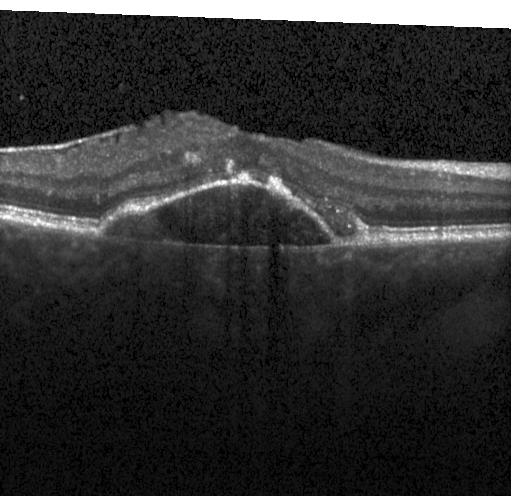 A choroidal neovascular membrane.